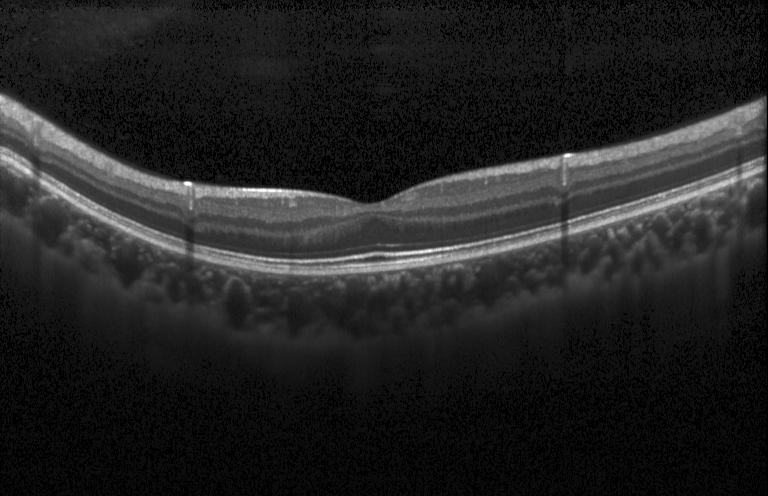 Macular scan, SD-OCT, OCT line scan. OCT finding: no choroidal neovascularization, diabetic macular edema, or drusen.